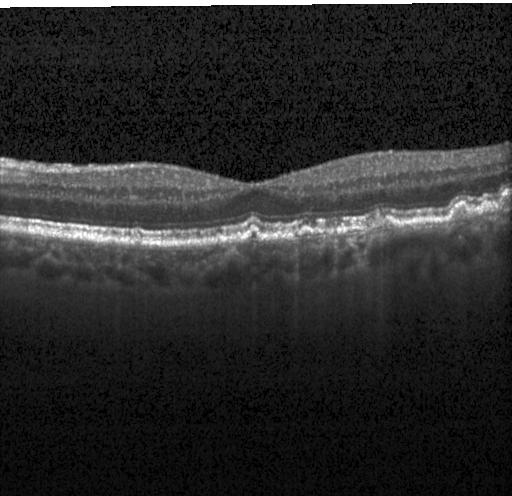

Heidelberg Spectralis · SD-OCT · optical coherence tomography scan.
This B-scan demonstrates drusen.